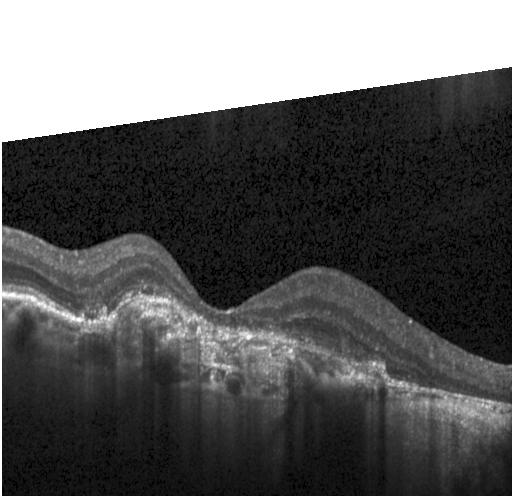 OCT line scan. Acquired on a Heidelberg Spectralis. SD-OCT. Centered on the fovea. Choroidal neovascularization (CNV).